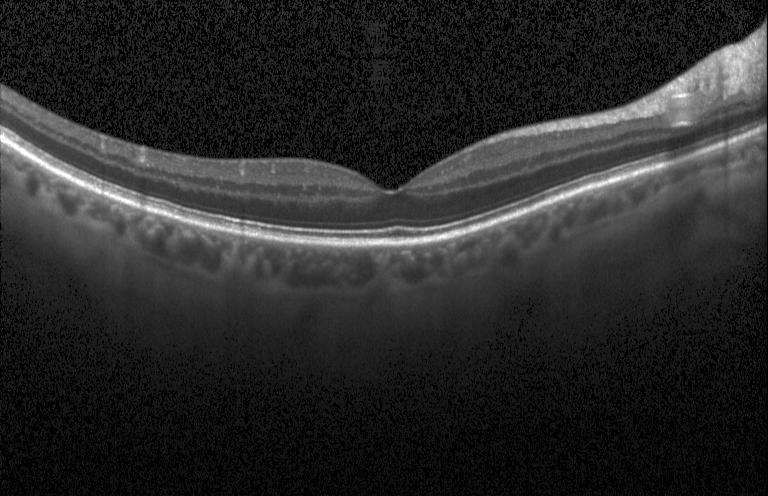

Optical coherence tomography scan, fovea-centered, instrument: Heidelberg Spectralis
Macular OCT: no choroidal neovascularization, diabetic macular edema, or drusen.